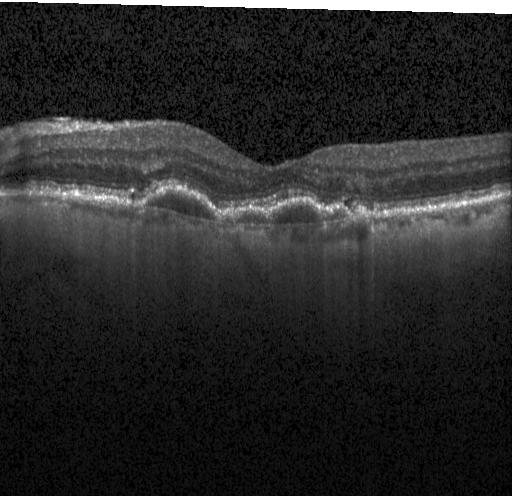
Fovea-centered. Optical coherence tomography B-scan
Finding: a choroidal neovascular membrane.